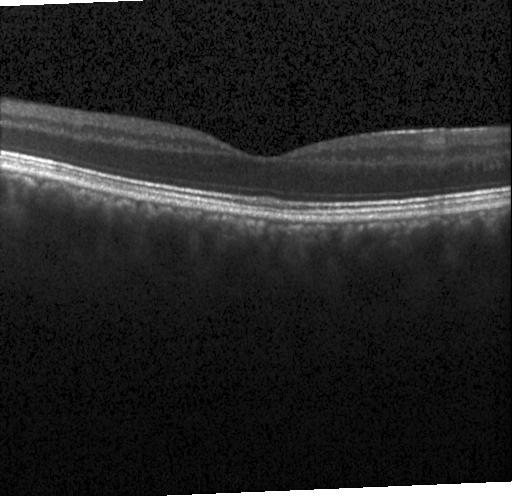
Assessment: no choroidal neovascularization, diabetic macular edema, or drusen.